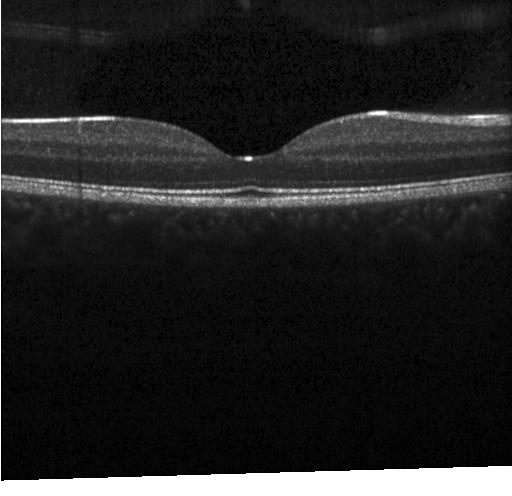 Retinal OCT B-scan, macular scan.
Assessment: no evidence of choroidal neovascularization, diabetic macular edema, or drusen.